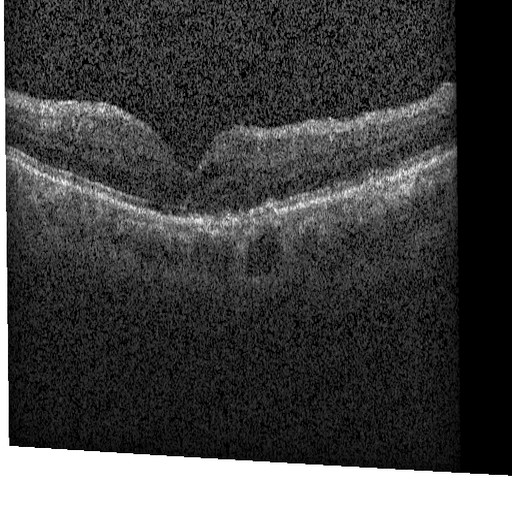

Centered on the fovea · acquired on a Heidelberg Spectralis · retinal OCT B-scan · spectral-domain OCT — Assessment: diabetic macular edema (DME).